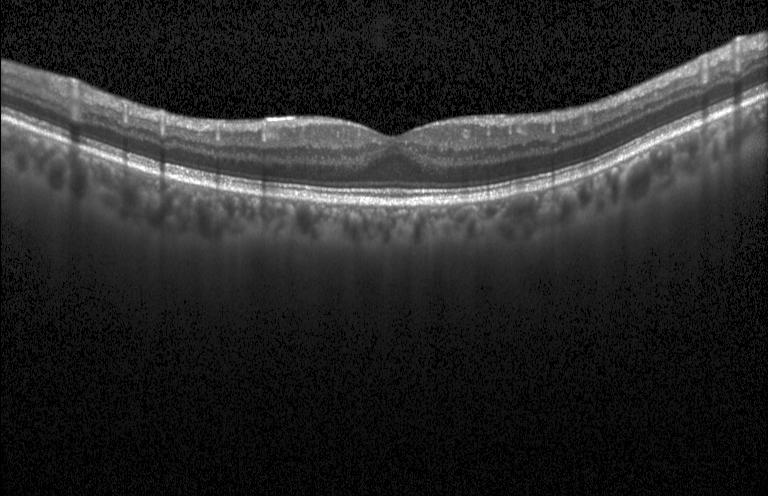
OCT line scan.
Finding: no choroidal neovascularization, diabetic macular edema, or drusen.